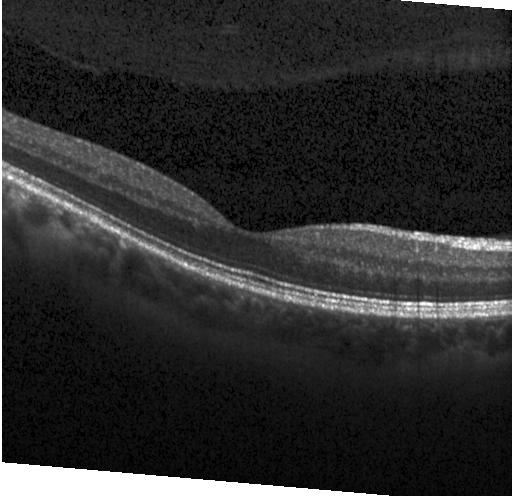

Heidelberg Spectralis · optical coherence tomography B-scan — Dx: neither CNV, DME, nor drusen.